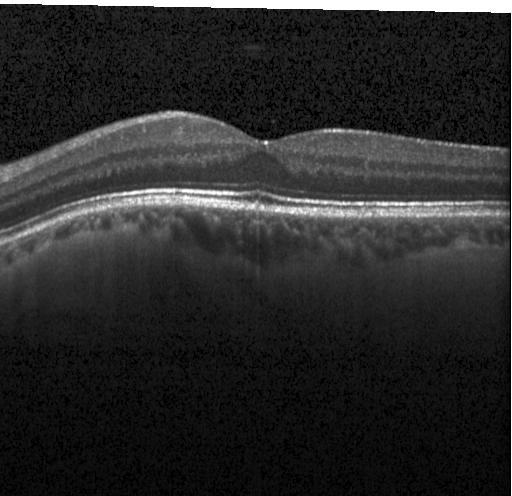

This B-scan demonstrates neither choroidal neovascularization, diabetic macular edema, nor drusen.